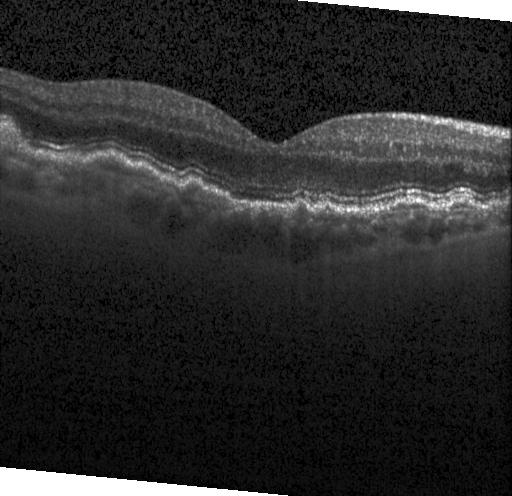

Finding: sub-RPE drusenoid deposits.